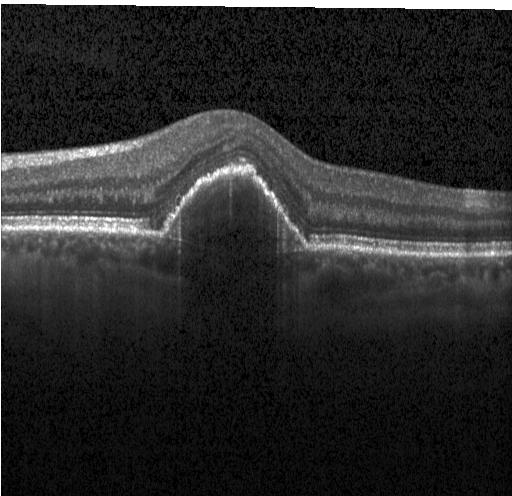
Optical coherence tomography B-scan, spectral-domain OCT — Macular OCT: choroidal neovascularization (CNV).